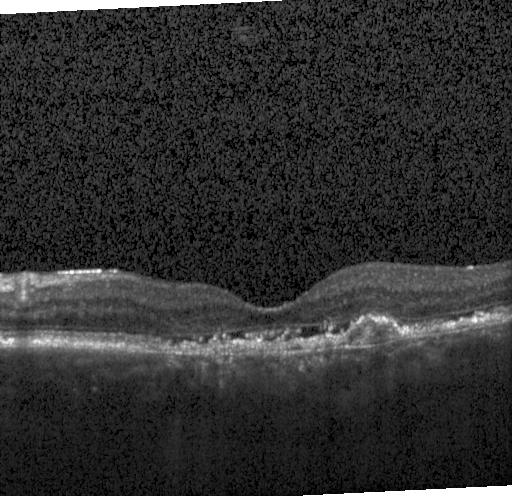
Retinal OCT cross-section. Finding: choroidal neovascularization (CNV).